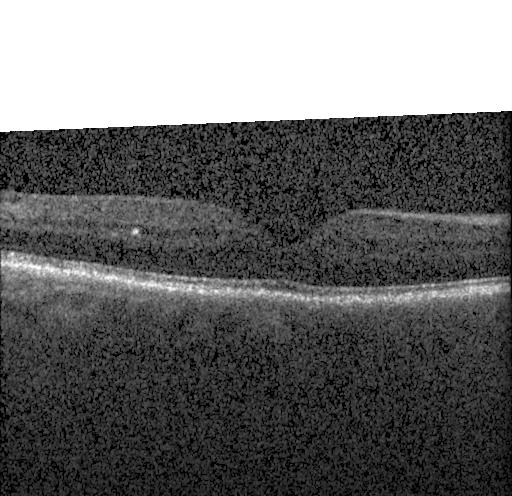 Spectral-domain OCT · OCT line scan. The scan shows no choroidal neovascularization, diabetic macular edema, or drusen.